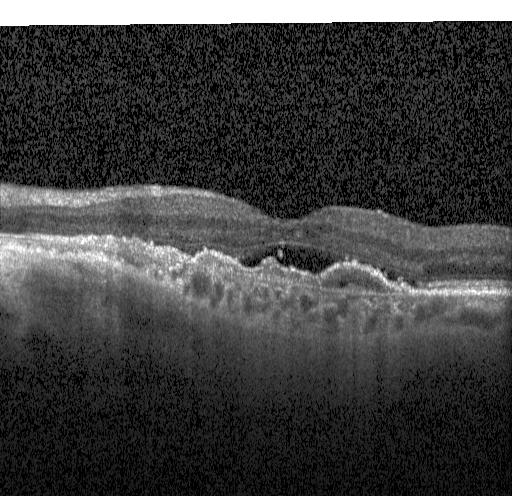
This B-scan demonstrates CNV.